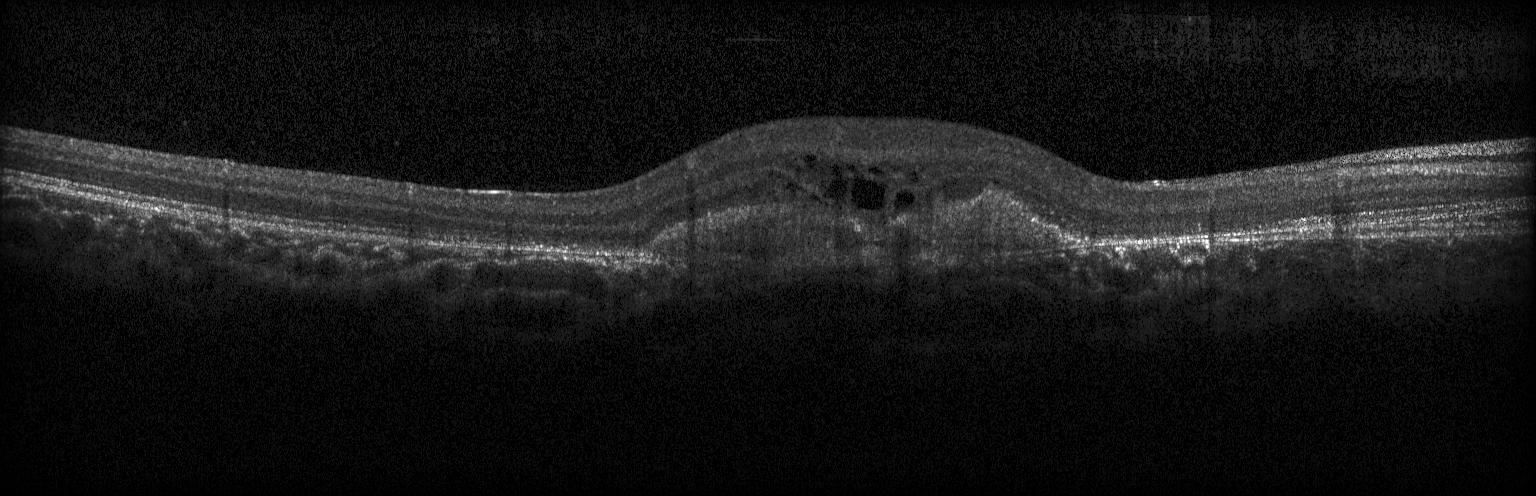
Impression: a choroidal neovascular membrane.